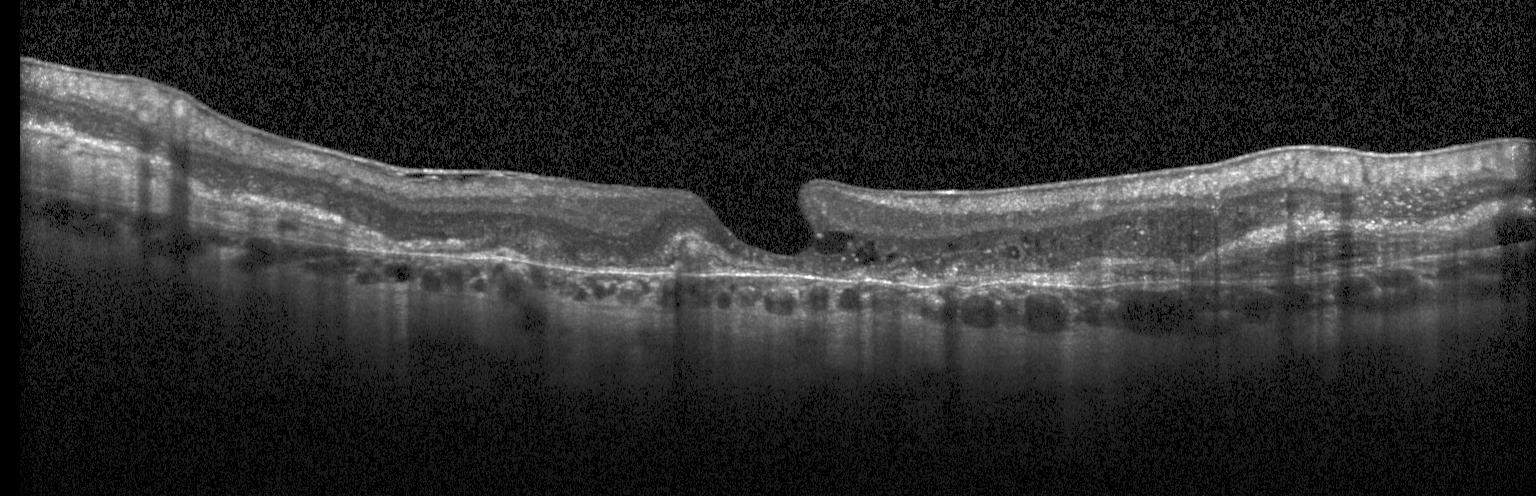 Through the macula; OCT B-scan; spectral-domain optical coherence tomography; acquired on a Heidelberg Spectralis — Finding: a choroidal neovascular membrane.